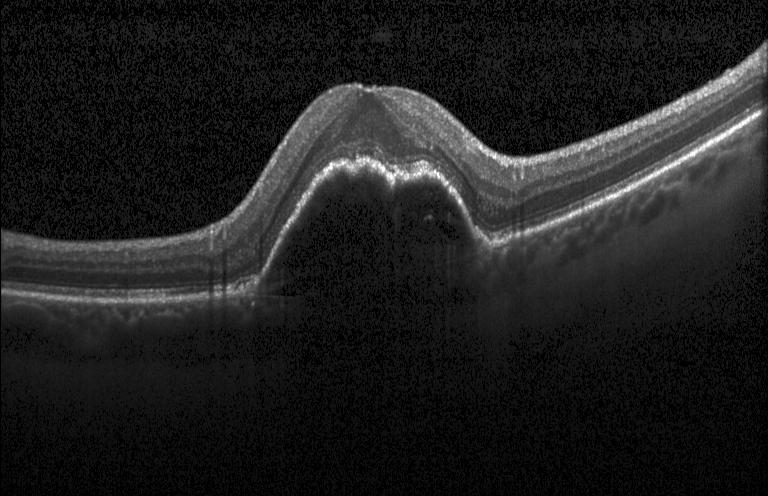 Diagnosis: CNV.